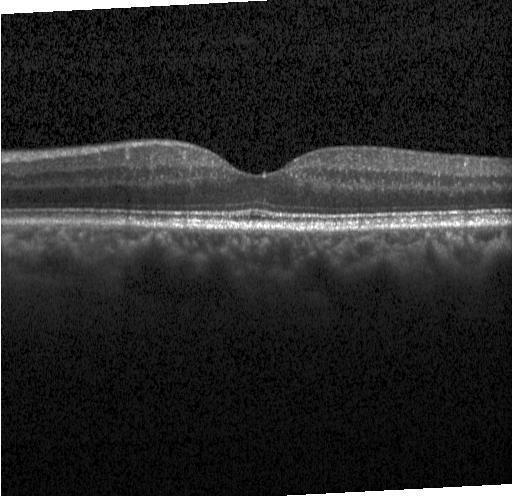

Finding: no choroidal neovascularization, diabetic macular edema, or drusen.